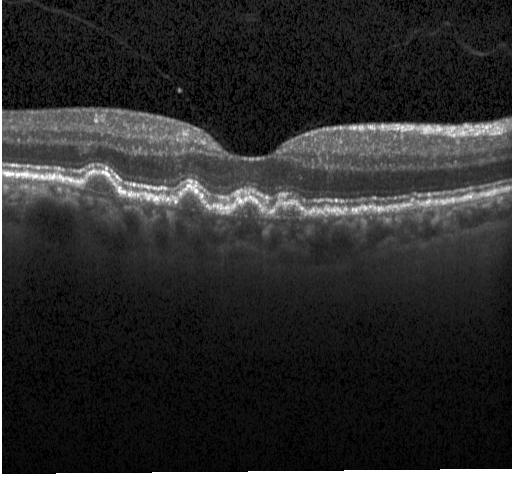 Finding: multiple drusen.